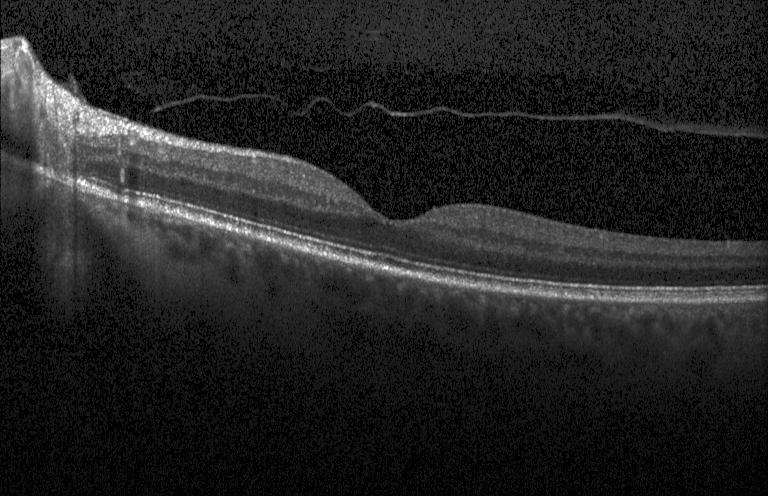
OCT B-scan showing neither choroidal neovascularization, diabetic macular edema, nor drusen.